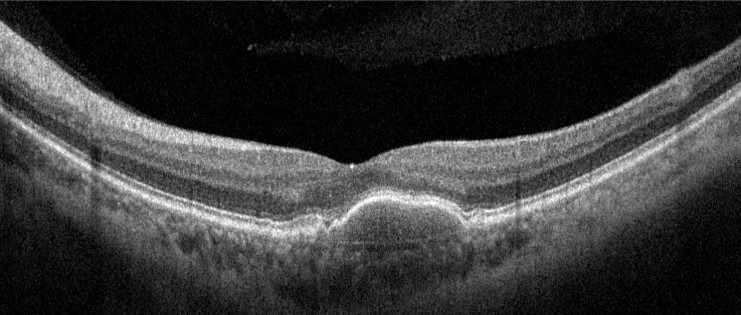
OCT B-scan. Assessment: age-related macular degeneration (AMD).